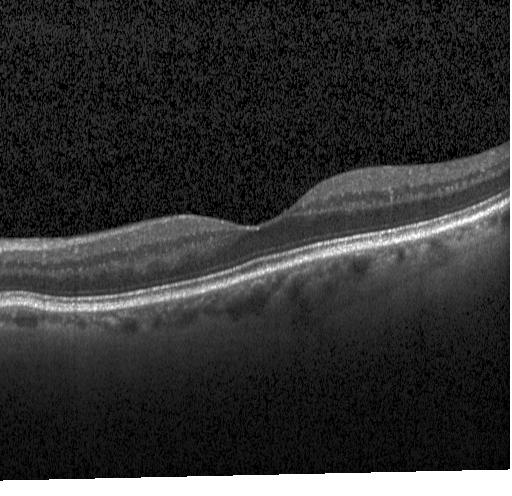
Retinal OCT cross-section, horizontal scan through the fovea, spectral-domain optical coherence tomography, Heidelberg Spectralis OCT system
Diagnosis: neither choroidal neovascularization, diabetic macular edema, nor drusen.